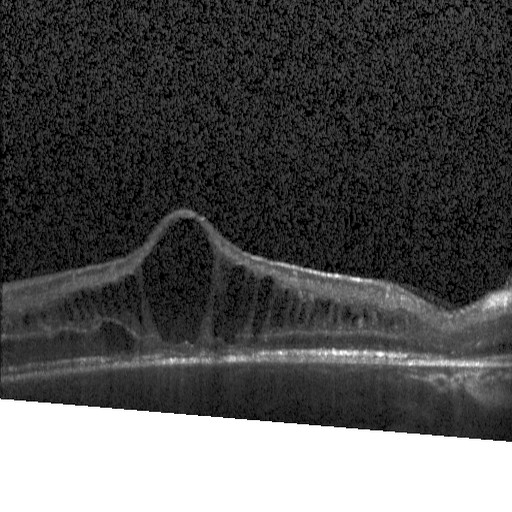

Through the macula, OCT B-scan, spectral-domain optical coherence tomography, Heidelberg Spectralis OCT system — This B-scan demonstrates DME.